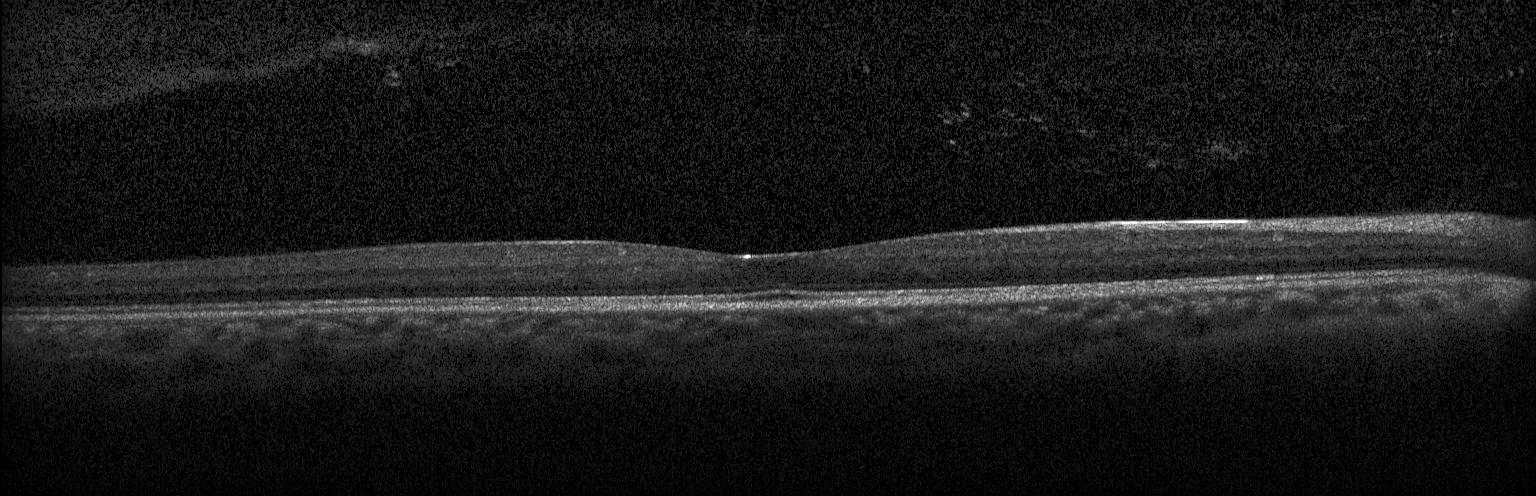 OCT B-scan showing no CNV, no DME, and no drusen.